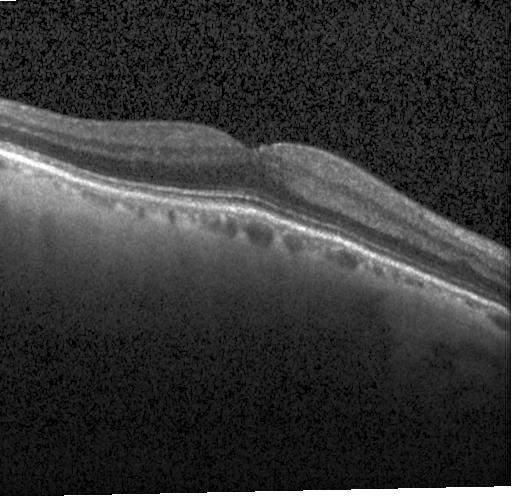 Diagnosis: no evidence of choroidal neovascularization, diabetic macular edema, or drusen.